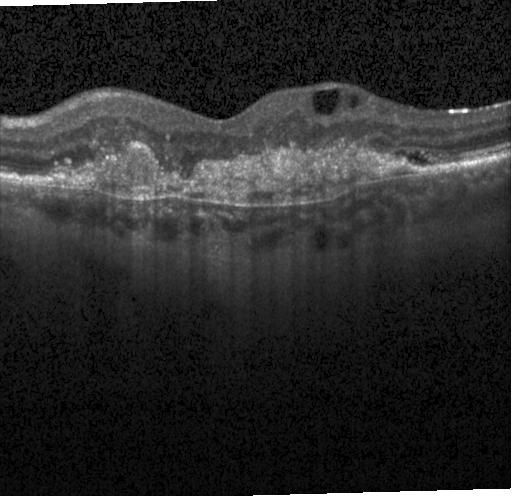 OCT B-scan showing CNV.